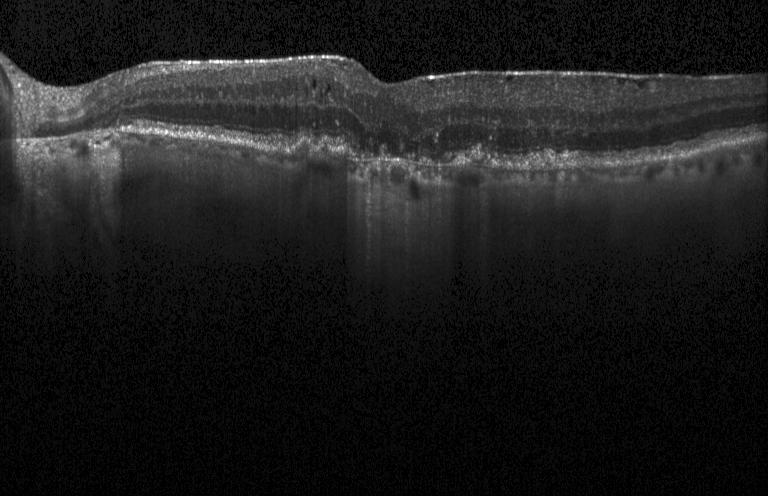 Macular scan. Instrument: Heidelberg Spectralis. Optical coherence tomography scan — Diagnosis: CNV.